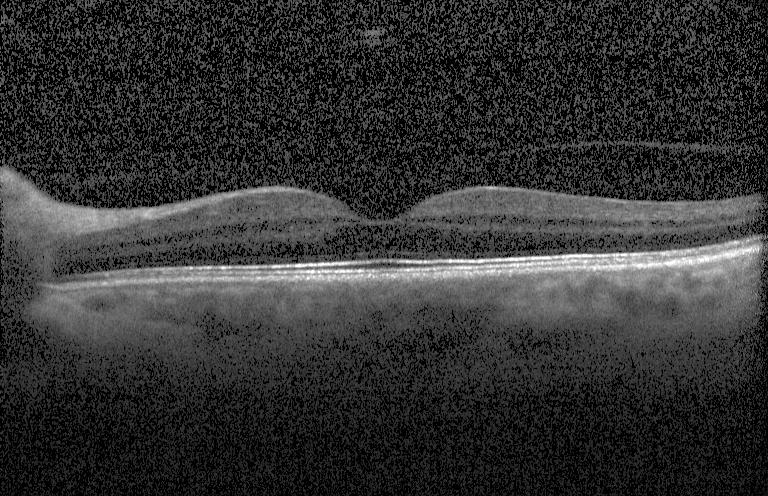
Macular OCT: no evidence of choroidal neovascularization, diabetic macular edema, or drusen.